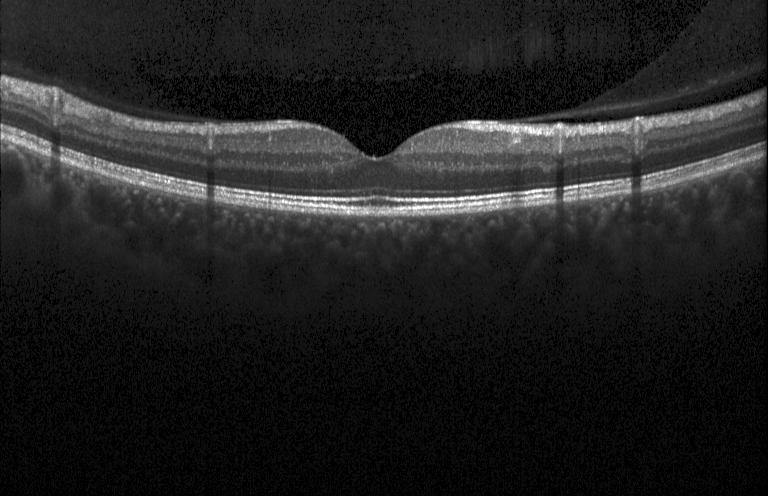
Centered on the fovea. Retinal OCT B-scan. Heidelberg Spectralis. SD-OCT. Diagnosis: no choroidal neovascularization, diabetic macular edema, or drusen.